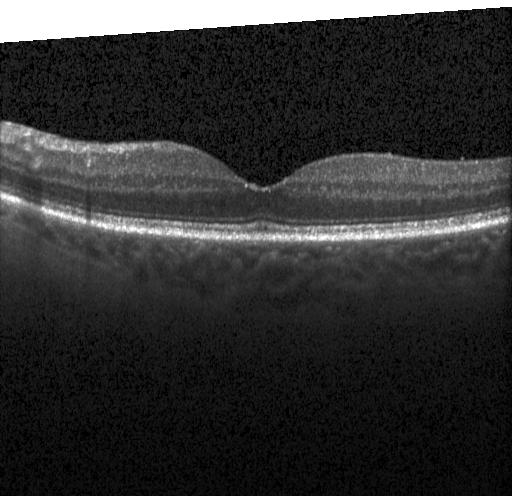

OCT line scan — OCT finding: no evidence of choroidal neovascularization, diabetic macular edema, or drusen.